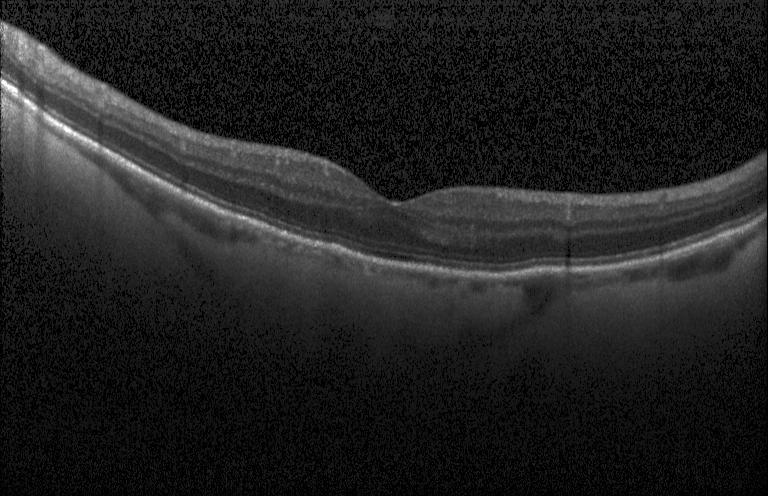 Spectral-domain OCT, OCT B-scan — Diagnosis: no evidence of choroidal neovascularization, diabetic macular edema, or drusen.